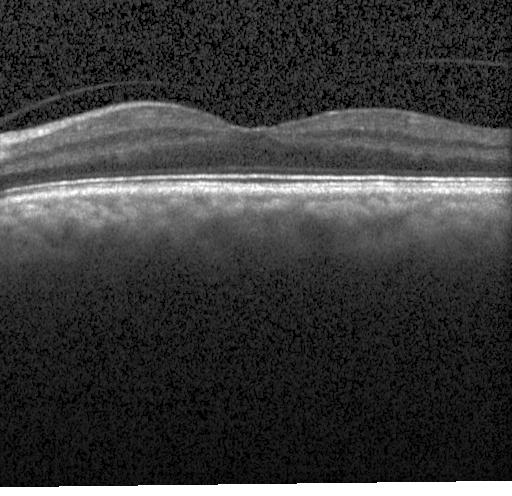

OCT B-scan. Diagnosis: no CNV, DME, or drusen.